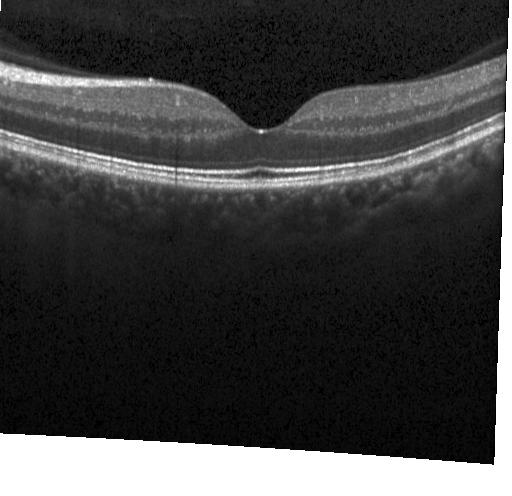

Retinal OCT B-scan. Spectral-domain optical coherence tomography. Acquired on a Heidelberg Spectralis. Centered on the fovea. Macular OCT: no evidence of CNV, DME, or drusen.